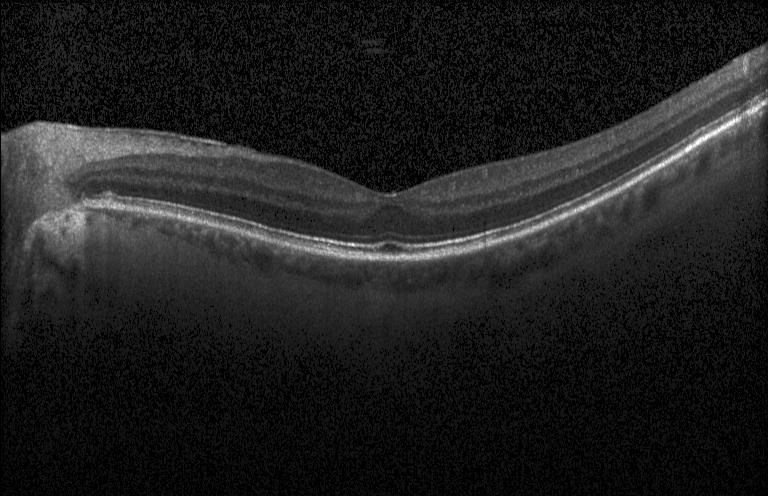 Centered on the fovea · Heidelberg Spectralis OCT system · OCT B-scan — Impression: no CNV, DME, or drusen.